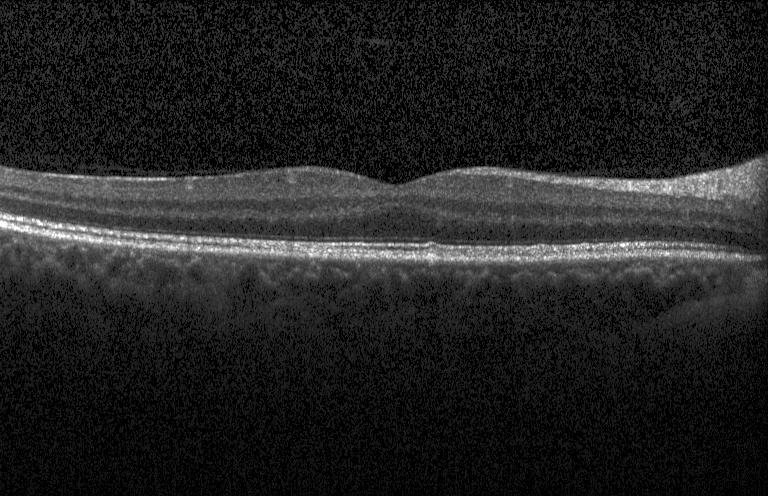 Optical coherence tomography scan. Impression: no CNV, DME, or drusen.